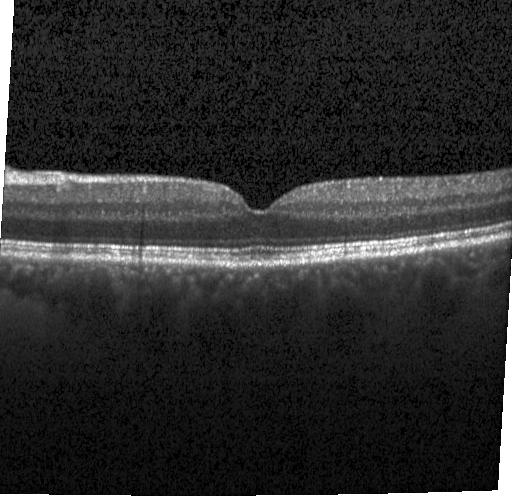

The scan shows no CNV, DME, or drusen.